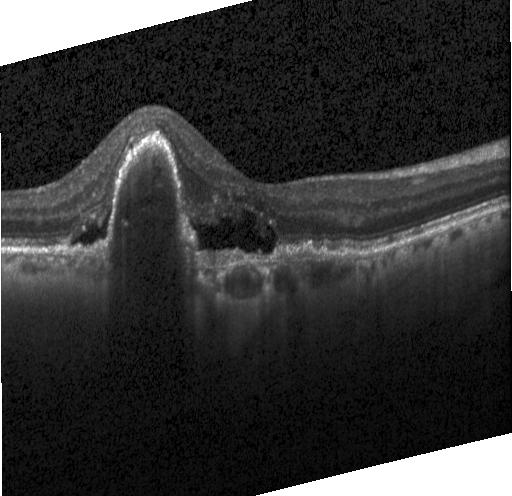
Optical coherence tomography scan · spectral-domain optical coherence tomography · acquired on a Heidelberg Spectralis
The scan shows a choroidal neovascular membrane.